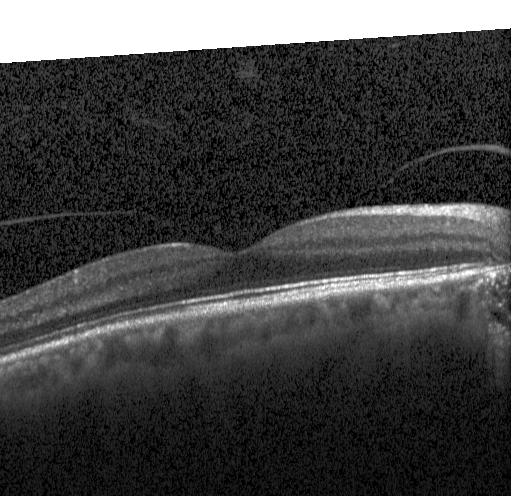

OCT line scan.
Diagnosis: no choroidal neovascularization, no diabetic macular edema, and no drusen.